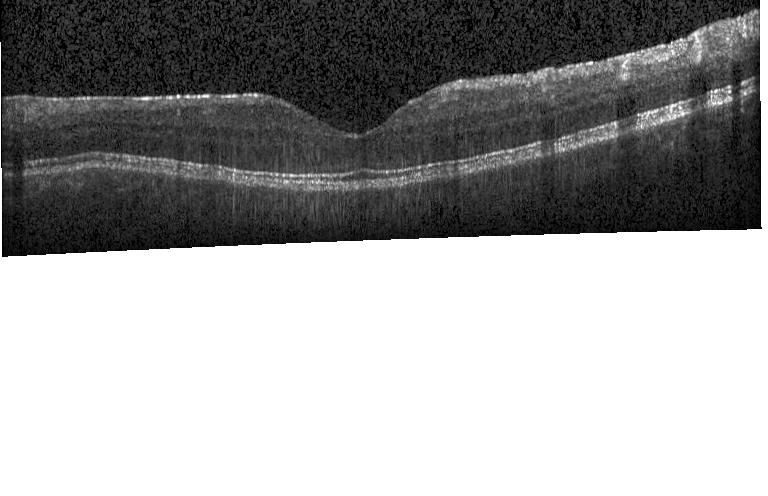

Diagnosis: no CNV, DME, or drusen.